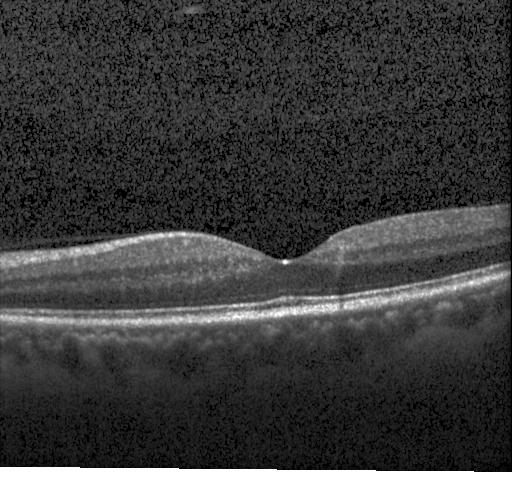
Macular scan · Heidelberg Spectralis · optical coherence tomography scan · SD-OCT. This B-scan demonstrates no CNV, no DME, and no drusen.